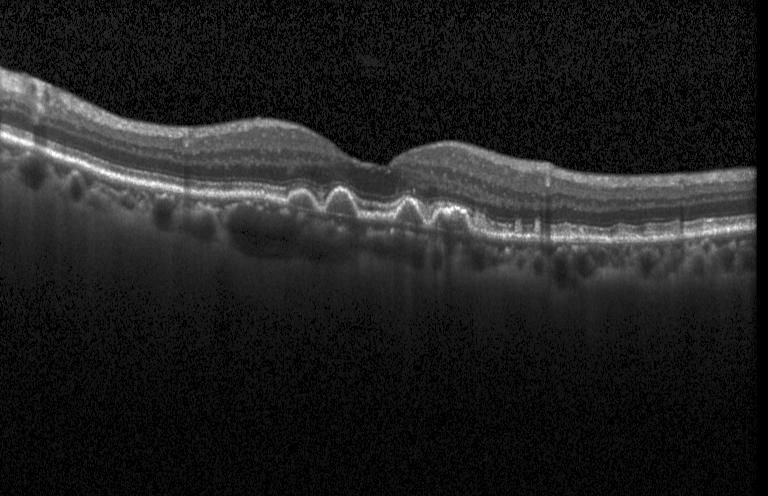
OCT line scan — Impression: sub-RPE drusenoid deposits.